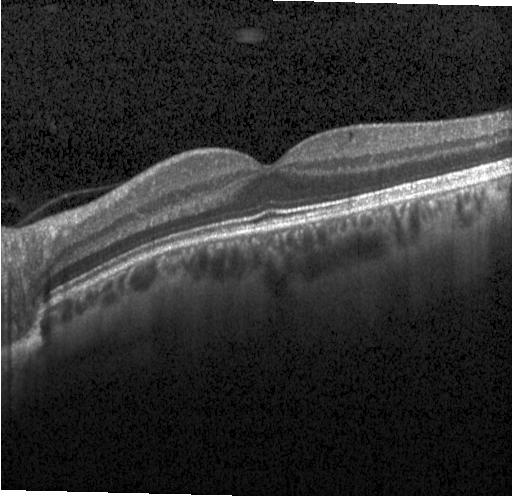

Finding: neither choroidal neovascularization, diabetic macular edema, nor drusen.